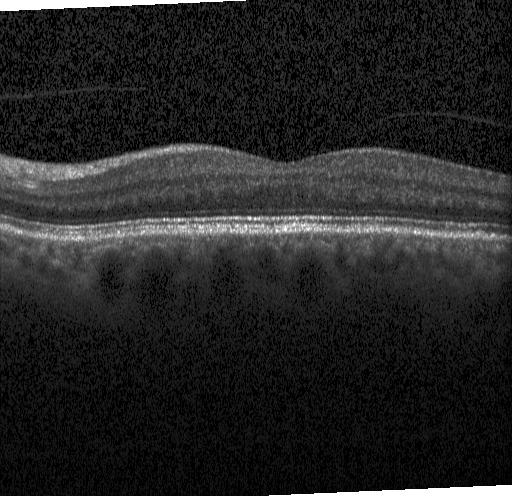 Finding: no evidence of choroidal neovascularization, diabetic macular edema, or drusen.